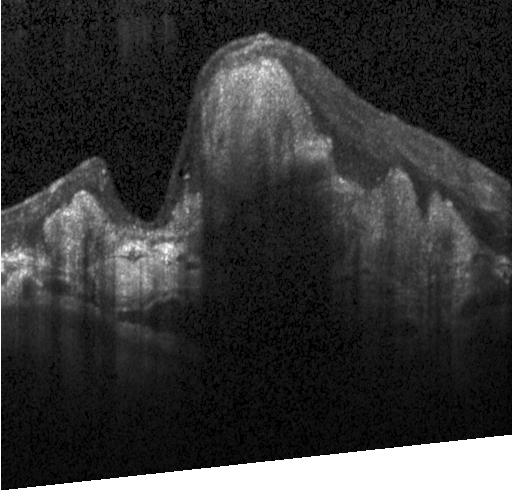 Finding: choroidal neovascularization.